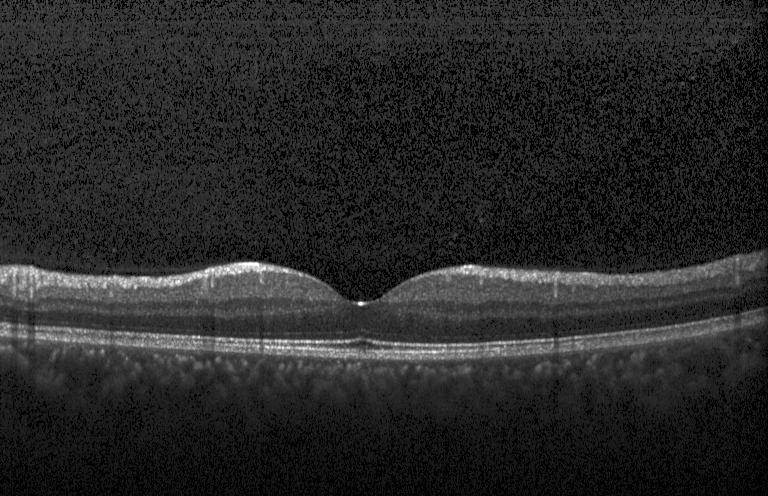 OCT B-scan · instrument: Heidelberg Spectralis
Diagnosis: no CNV, no DME, and no drusen.